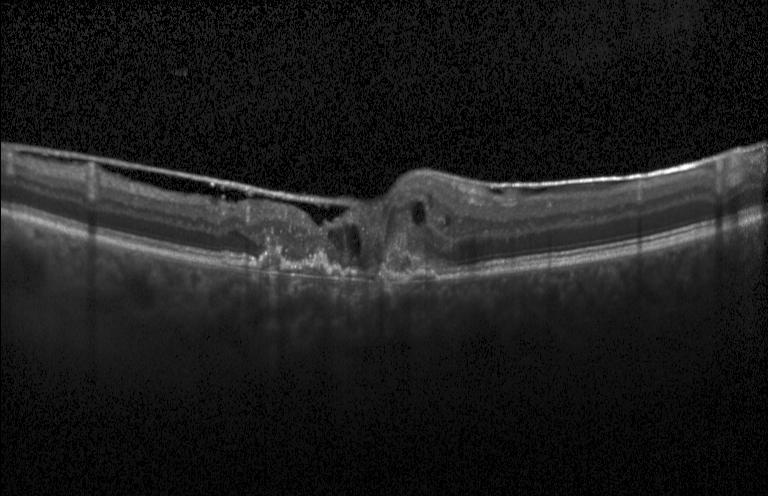
Finding: CNV.